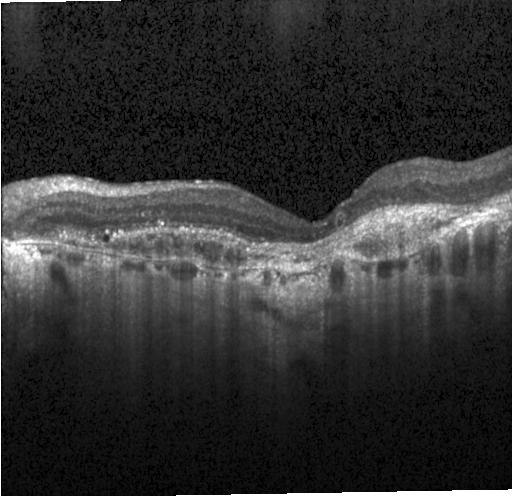 The scan shows choroidal neovascularization.